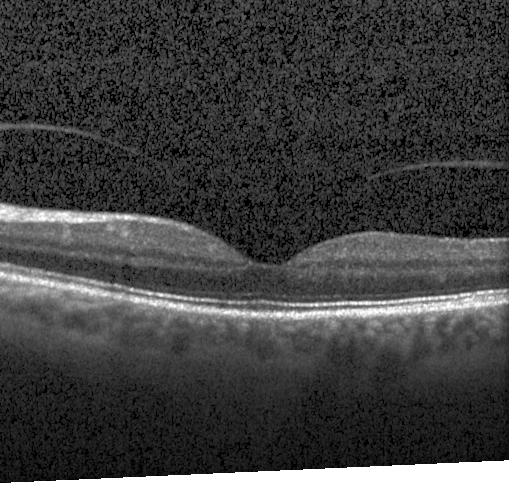
Retinal OCT B-scan · Heidelberg Spectralis OCT system.
Impression: no CNV, no DME, and no drusen.